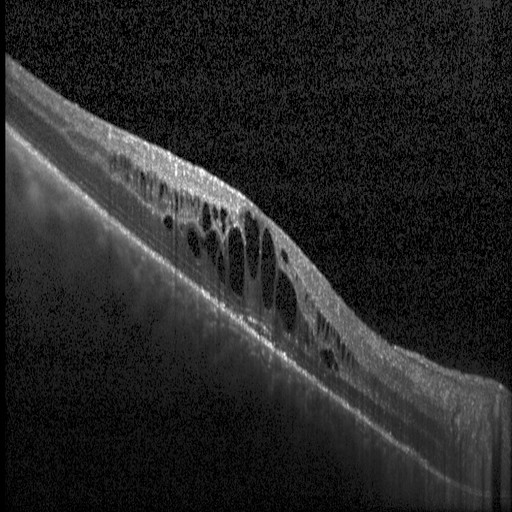

Impression: diabetic macular edema.